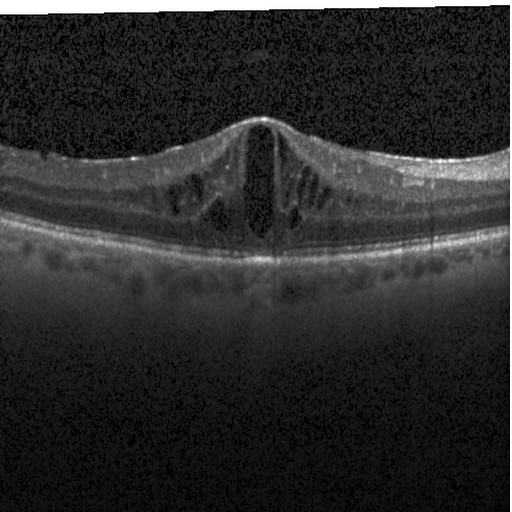
Acquired on a Heidelberg Spectralis. Horizontal scan through the fovea. Spectral-domain optical coherence tomography. Optical coherence tomography B-scan.
Assessment: diabetic macular edema.